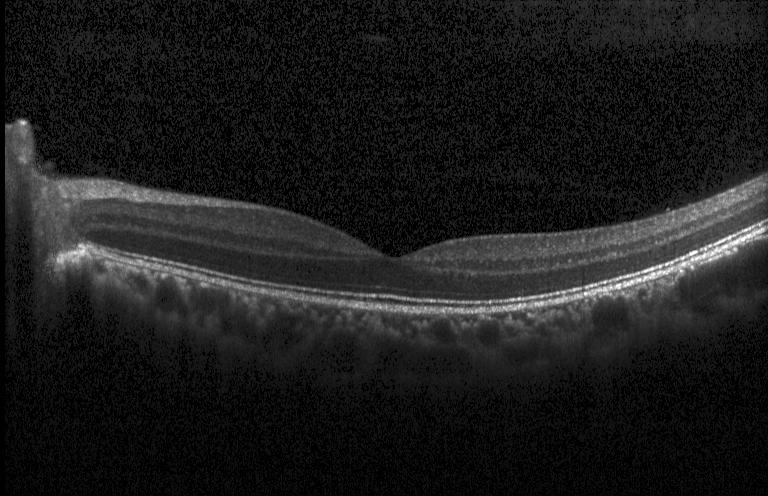

Diagnosis: no evidence of choroidal neovascularization, diabetic macular edema, or drusen.